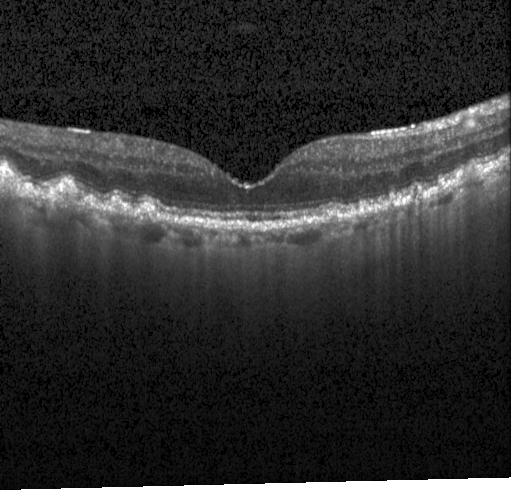
Optical coherence tomography B-scan · spectral-domain OCT.
Impression: sub-RPE drusenoid deposits.